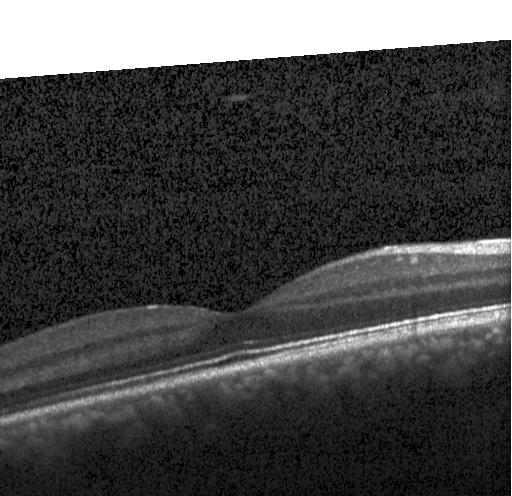

Impression: no evidence of CNV, DME, or drusen.